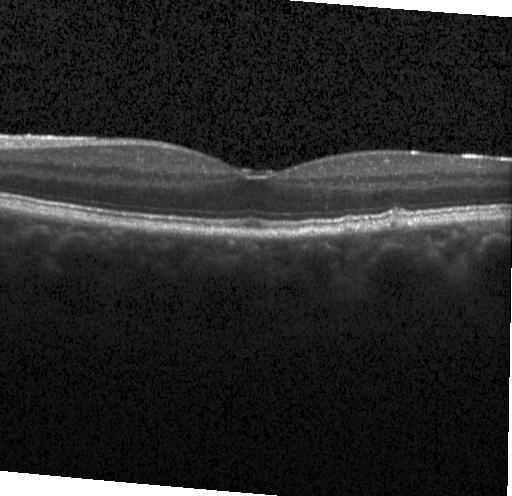 Macular OCT: multiple drusen.